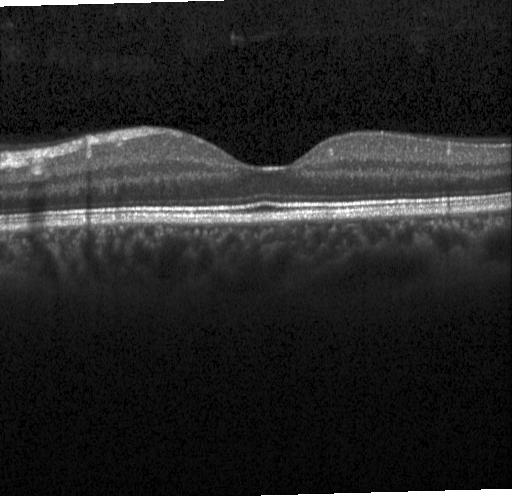 Centered on the fovea, spectral-domain optical coherence tomography, OCT line scan, Heidelberg Spectralis OCT system — Assessment: no evidence of CNV, DME, or drusen.